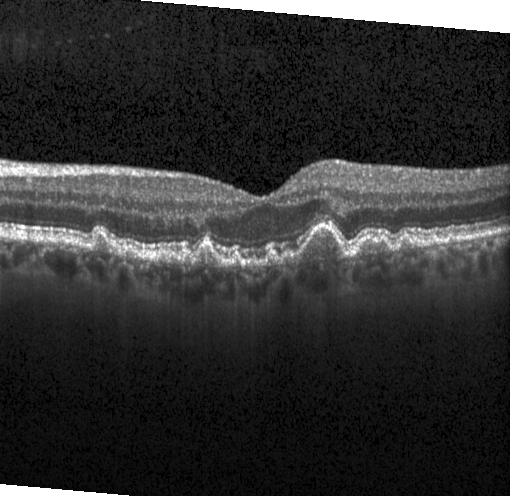
Retinal OCT B-scan; acquired on a Heidelberg Spectralis
Finding: sub-RPE drusenoid deposits.